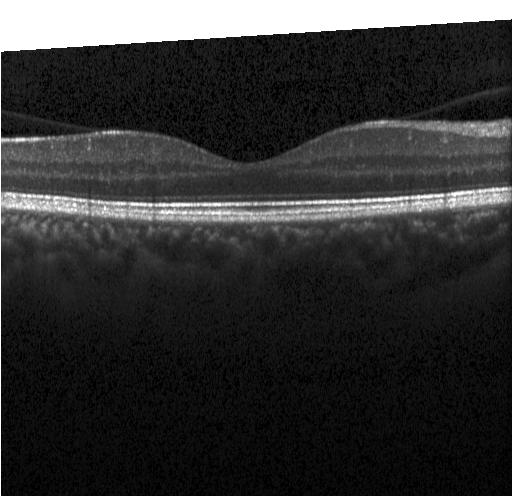

OCT line scan · instrument: Heidelberg Spectralis
Finding: no choroidal neovascularization, diabetic macular edema, or drusen.